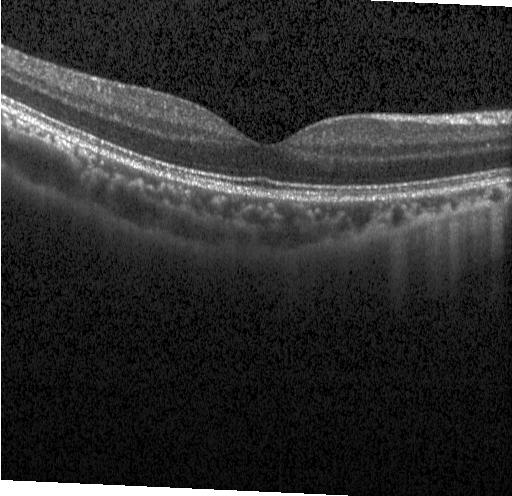 Diagnosis: no choroidal neovascularization, diabetic macular edema, or drusen.